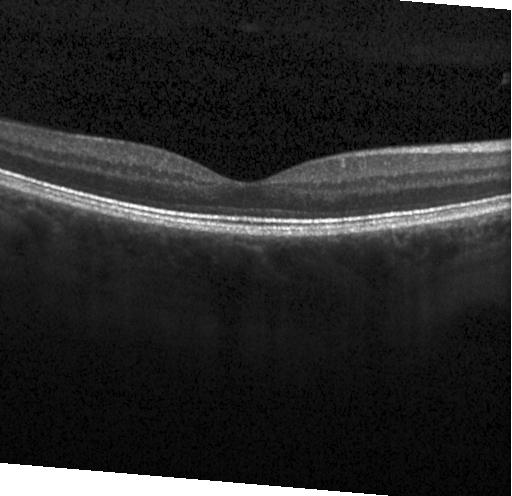
Impression: neither choroidal neovascularization, diabetic macular edema, nor drusen.